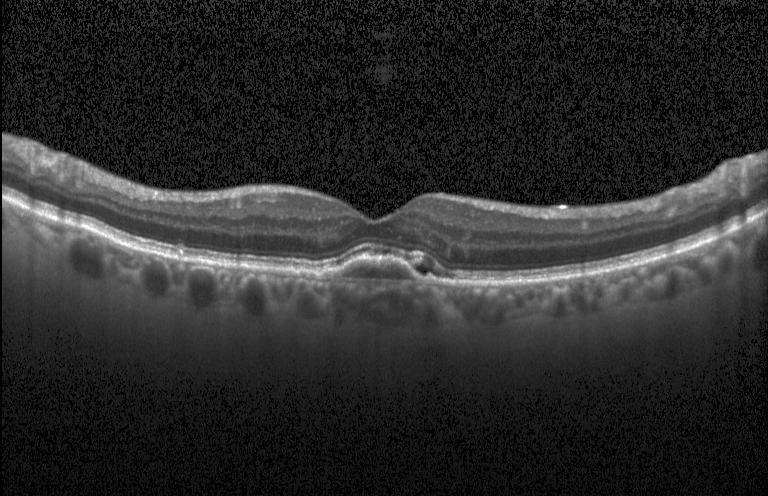
Retinal OCT B-scan. Spectral-domain optical coherence tomography. Horizontal scan through the fovea. Instrument: Heidelberg Spectralis
Macular OCT: a choroidal neovascular membrane.